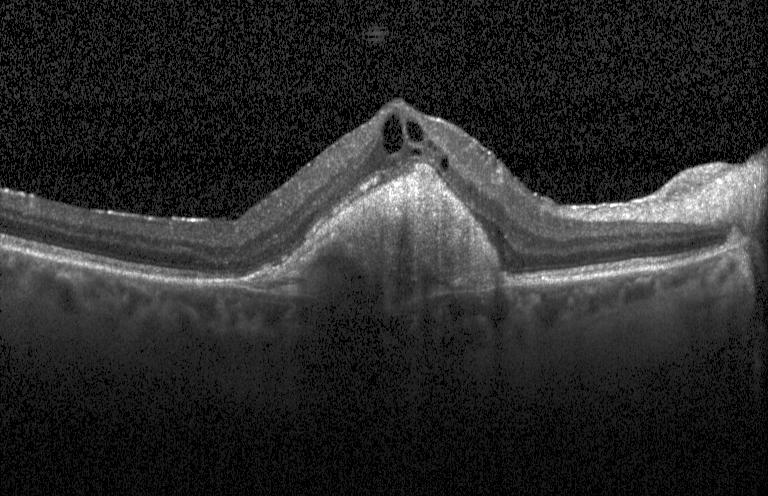

Spectral-domain OCT B-scan: CNV.